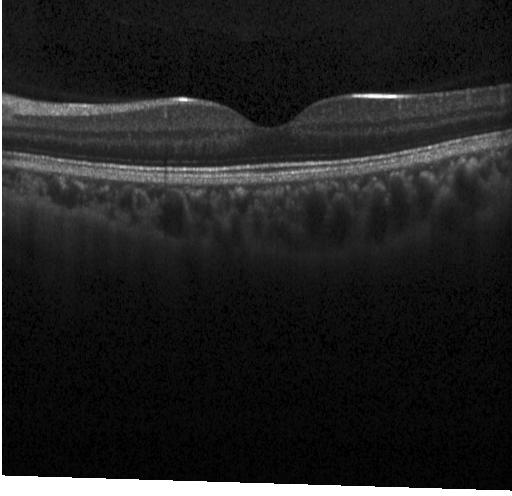
Assessment: no CNV, no DME, and no drusen.